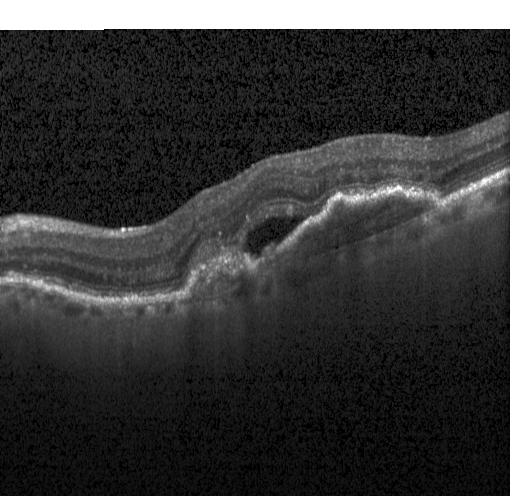
Spectral-domain OCT B-scan: CNV.